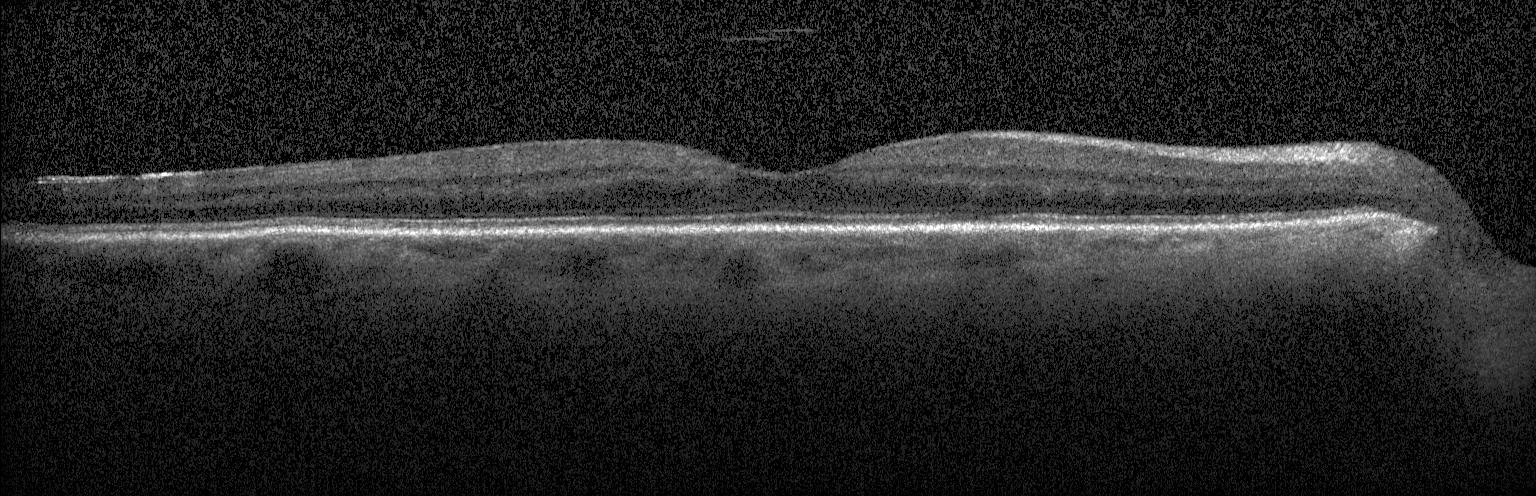

Diagnosis: no choroidal neovascularization, diabetic macular edema, or drusen.